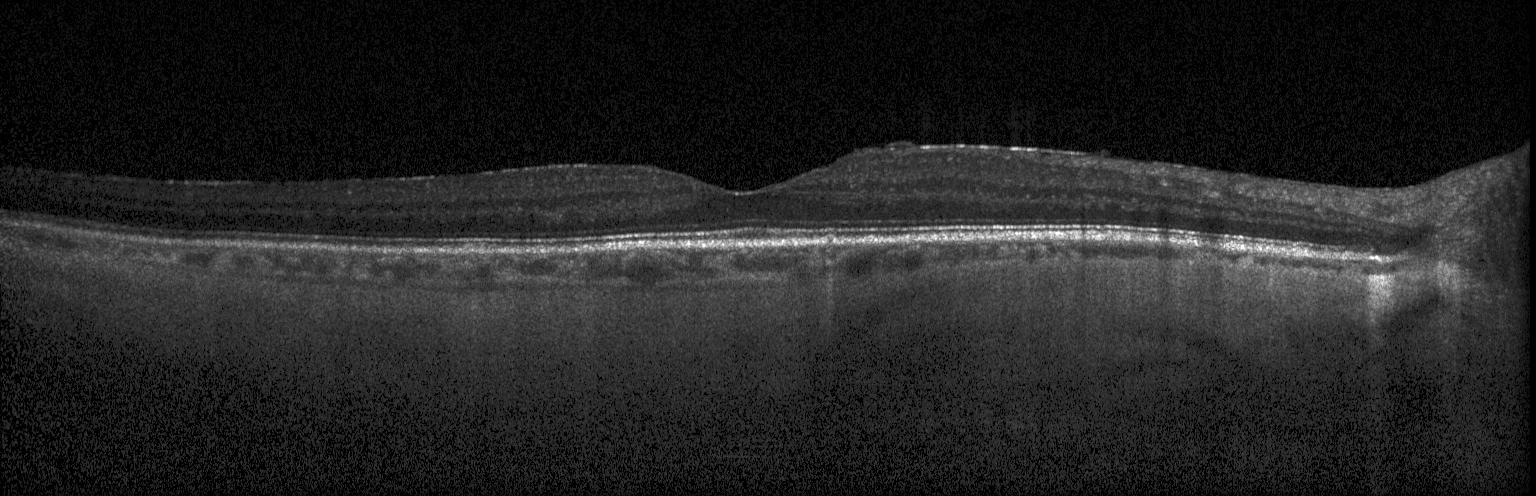

The scan shows neither choroidal neovascularization, diabetic macular edema, nor drusen.